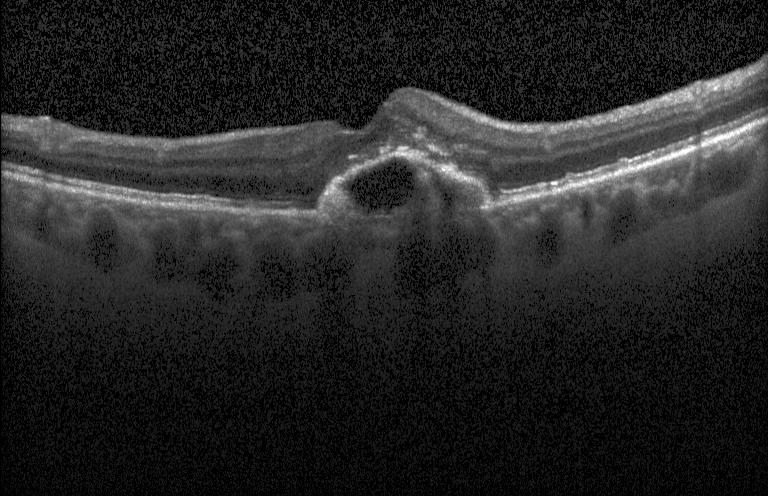 Horizontal scan through the fovea, optical coherence tomography scan, SD-OCT, Heidelberg Spectralis
A choroidal neovascular membrane.